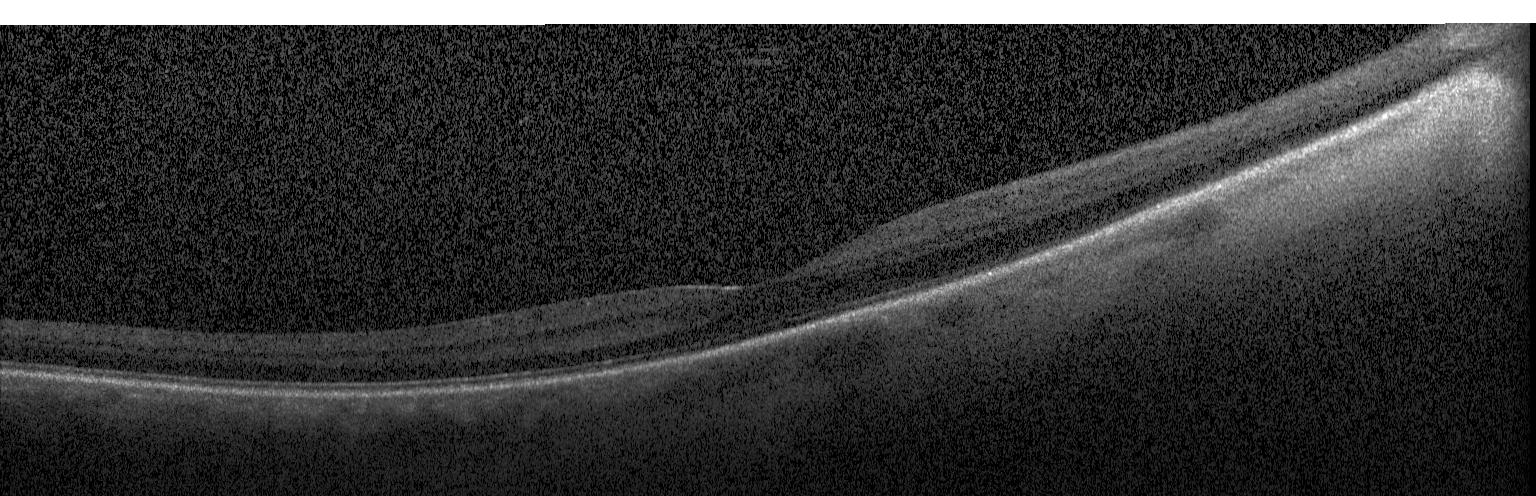
OCT scan showing no CNV, no DME, and no drusen.